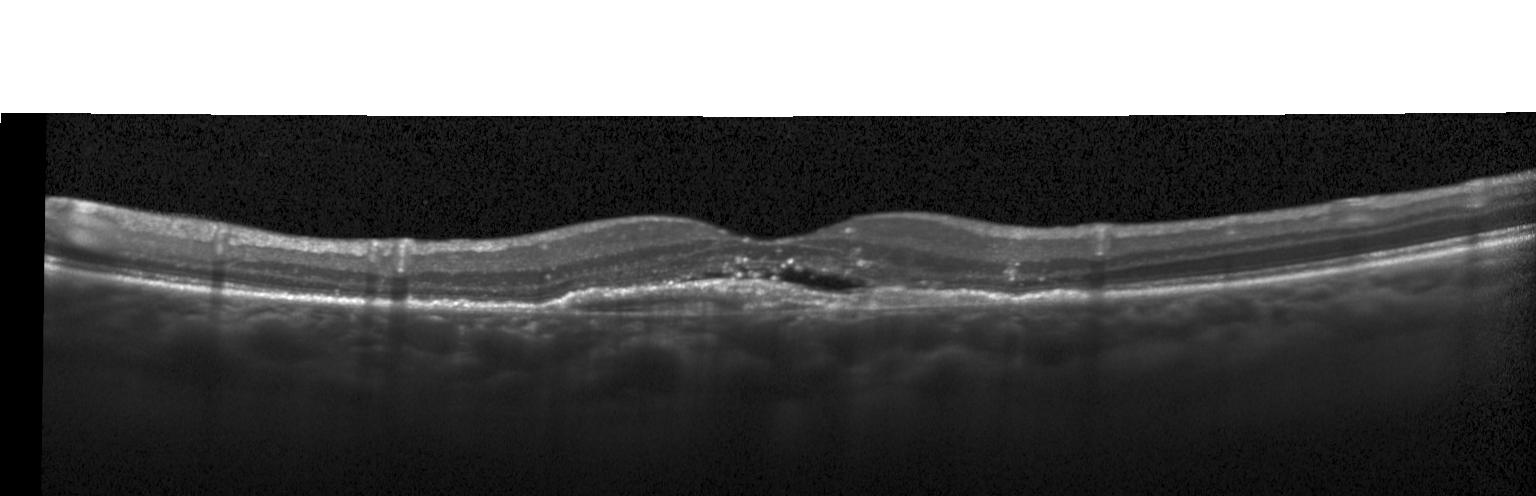

Heidelberg Spectralis. Optical coherence tomography B-scan. Spectral-domain OCT. Through the macula
This B-scan demonstrates a choroidal neovascular membrane.